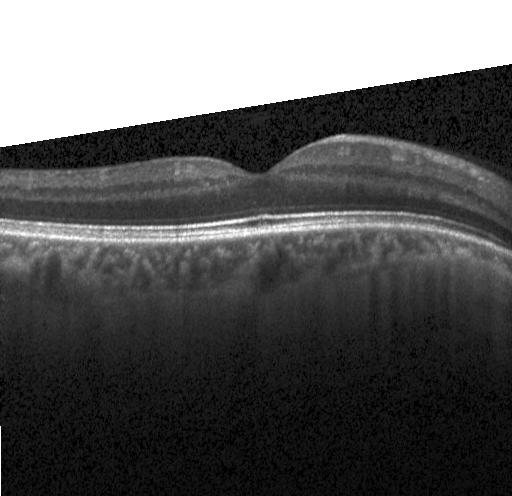

Retinal OCT B-scan · fovea-centered · SD-OCT — Finding: no evidence of choroidal neovascularization, diabetic macular edema, or drusen.